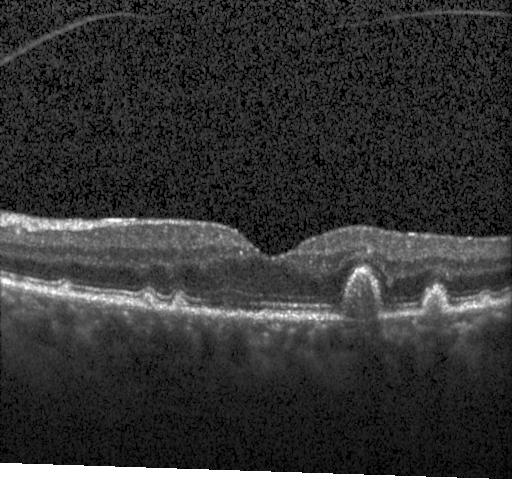 Optical coherence tomography B-scan; spectral-domain OCT — OCT finding: sub-RPE drusenoid deposits.